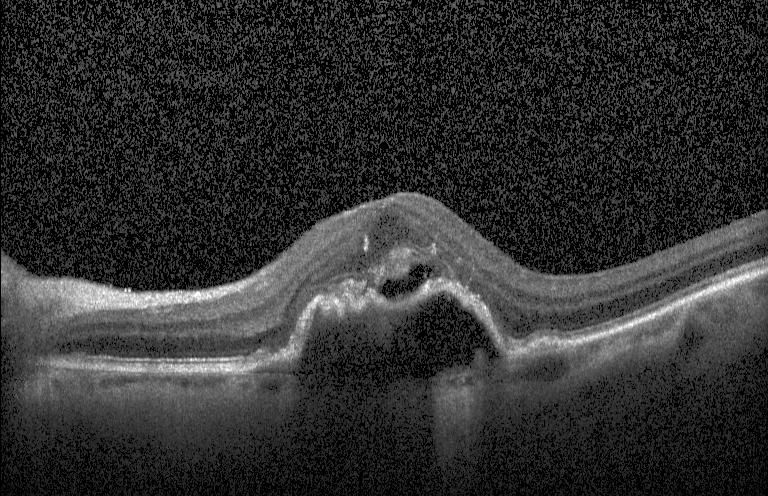 Heidelberg Spectralis OCT system · OCT B-scan · spectral-domain optical coherence tomography. Diagnosis: a choroidal neovascular membrane.